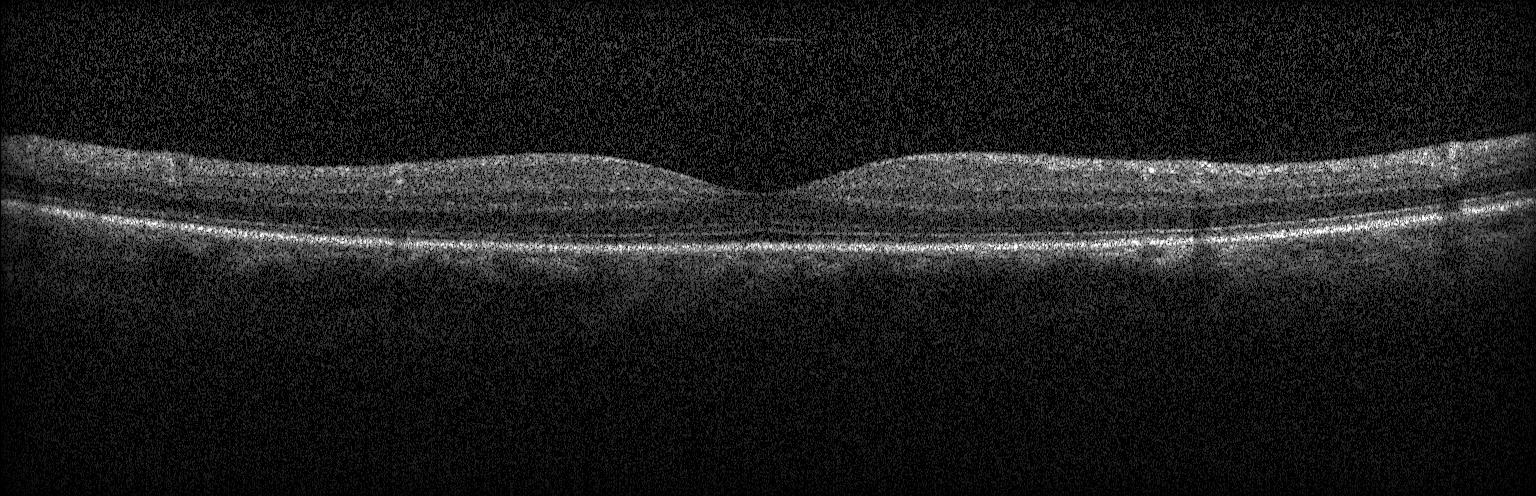

Centered on the fovea, Heidelberg Spectralis, retinal OCT cross-section
Finding: neither CNV, DME, nor drusen.